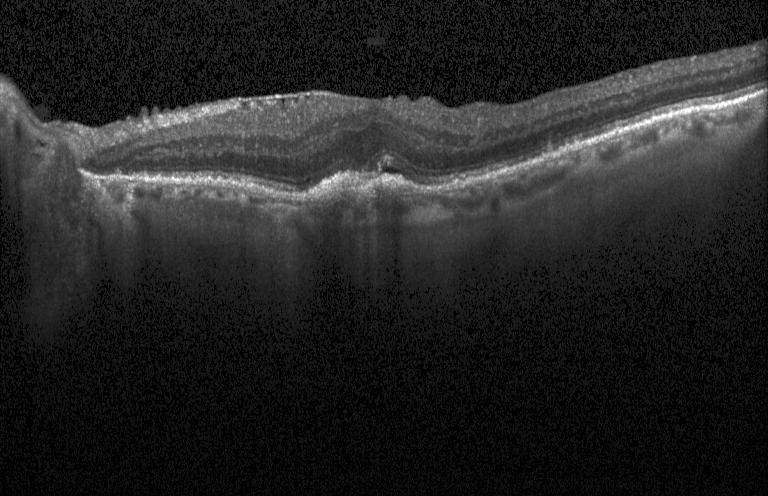
This B-scan demonstrates a choroidal neovascular membrane.